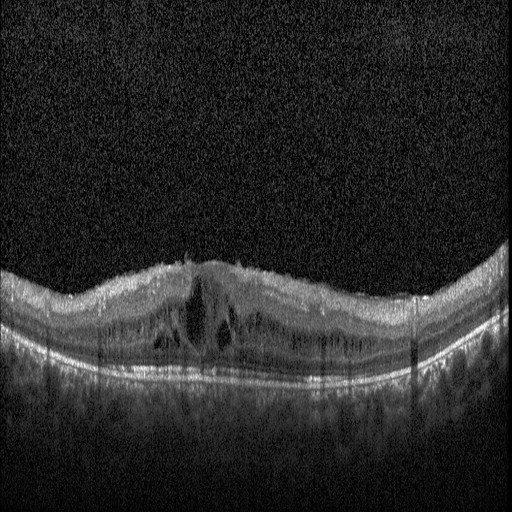 Assessment: DME.